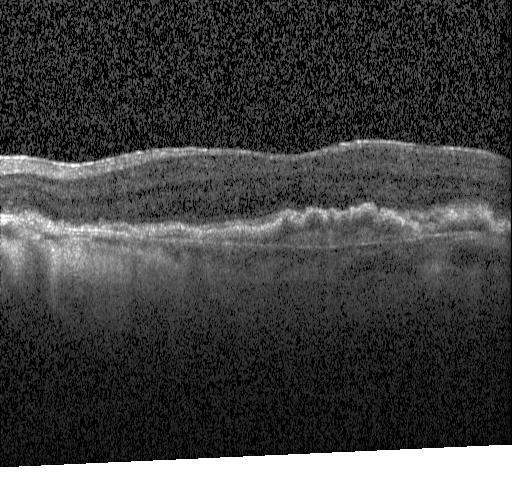
The scan shows a choroidal neovascular membrane.